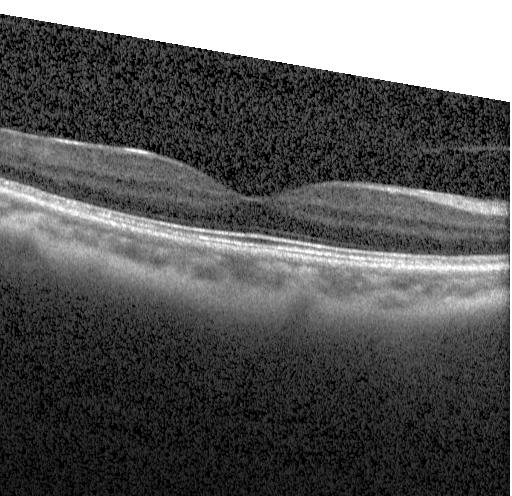 Impression: neither choroidal neovascularization, diabetic macular edema, nor drusen.